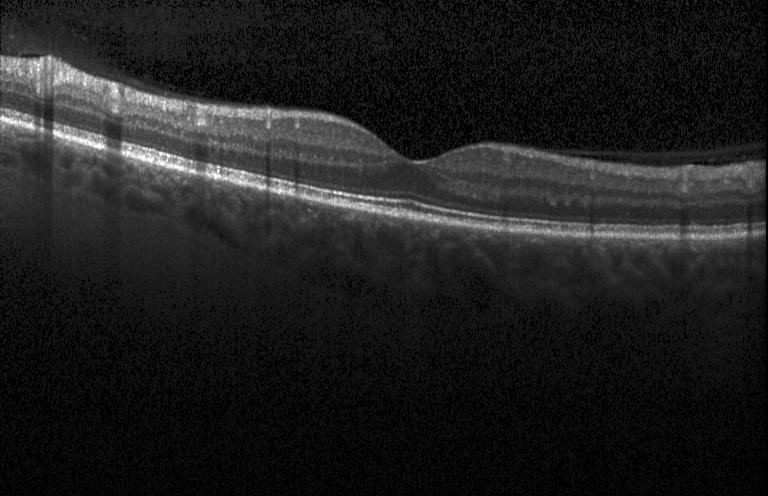 Spectral-domain OCT B-scan: no evidence of choroidal neovascularization, diabetic macular edema, or drusen.